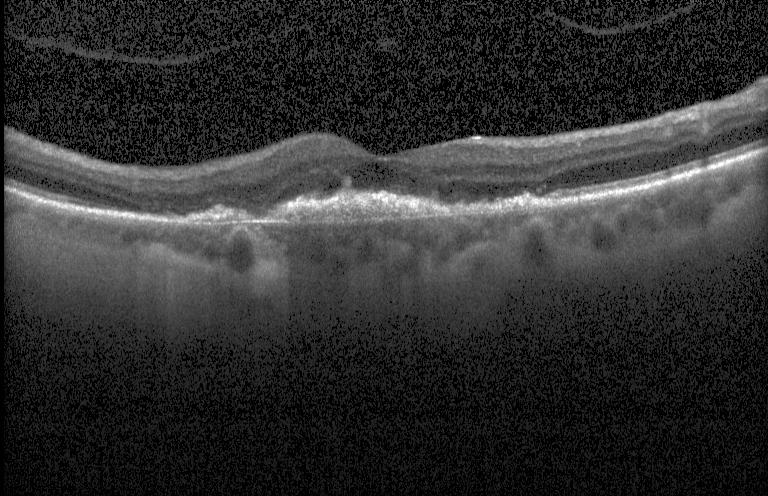
Retinal OCT B-scan. Spectral-domain OCT. Fovea-centered
Diagnosis: choroidal neovascularization.